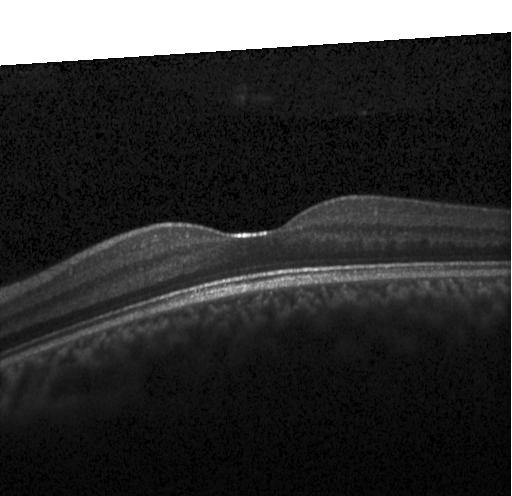 Optical coherence tomography B-scan.
The scan shows no CNV, no DME, and no drusen.